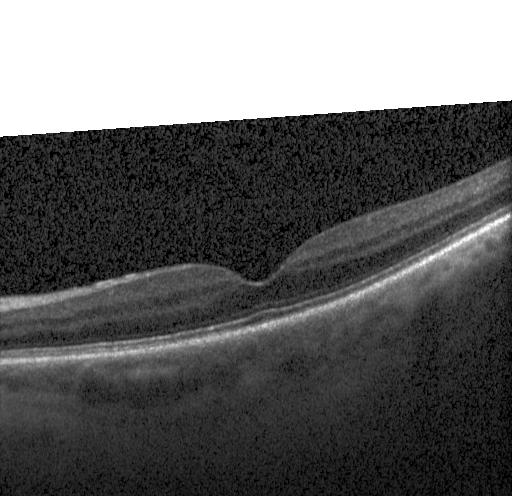 Impression: no choroidal neovascularization, diabetic macular edema, or drusen.